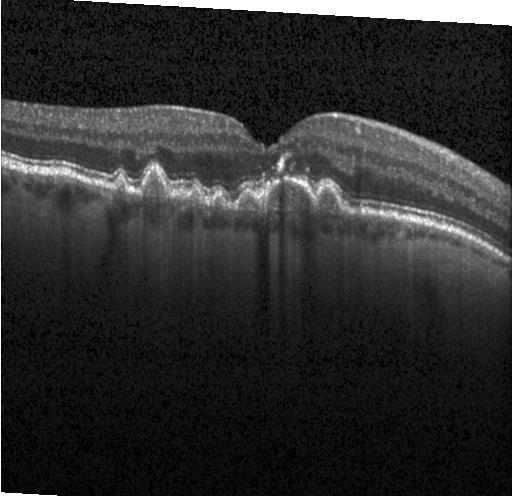
Acquired on a Heidelberg Spectralis; retinal OCT B-scan; fovea-centered.
Dx: sub-RPE drusenoid deposits.